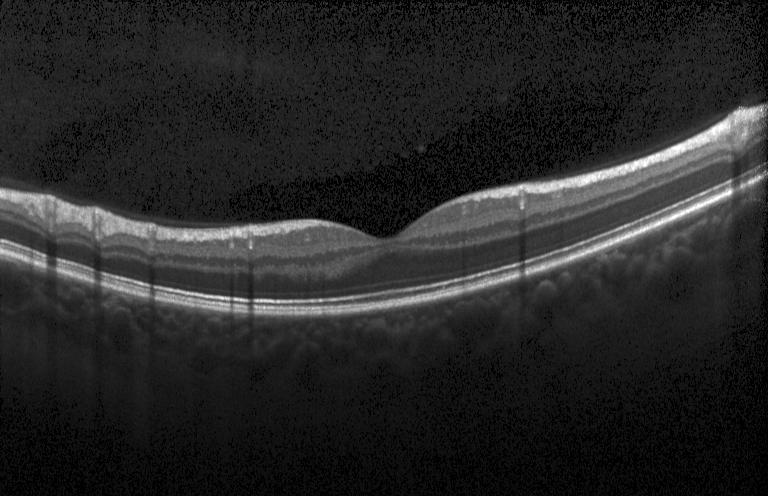

OCT line scan. Heidelberg Spectralis OCT system.
Finding: no choroidal neovascularization, no diabetic macular edema, and no drusen.